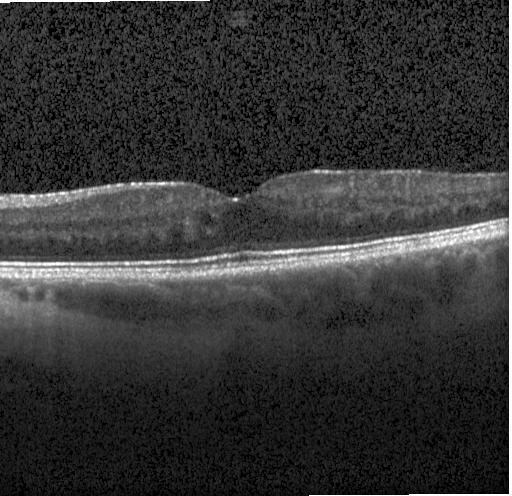 Macular OCT: neither choroidal neovascularization, diabetic macular edema, nor drusen.